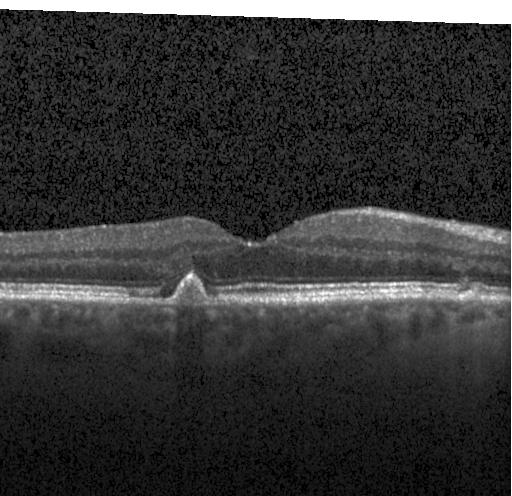
Dx: drusen.